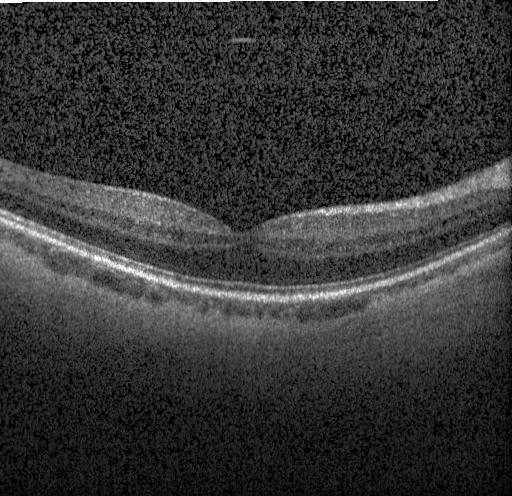 OCT scan showing no evidence of choroidal neovascularization, diabetic macular edema, or drusen.